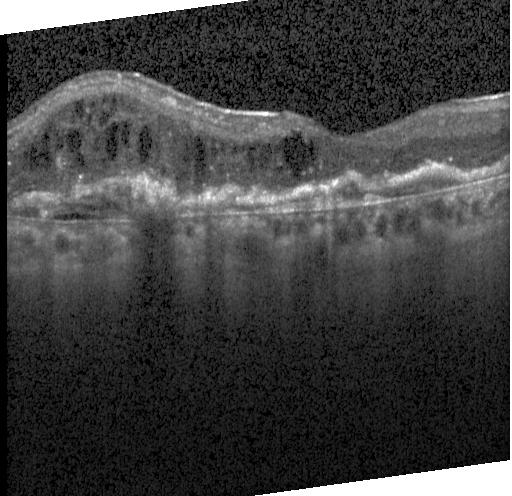
OCT B-scan. Spectral-domain OCT. Horizontal scan through the fovea. Heidelberg Spectralis OCT system.
Finding: CNV.